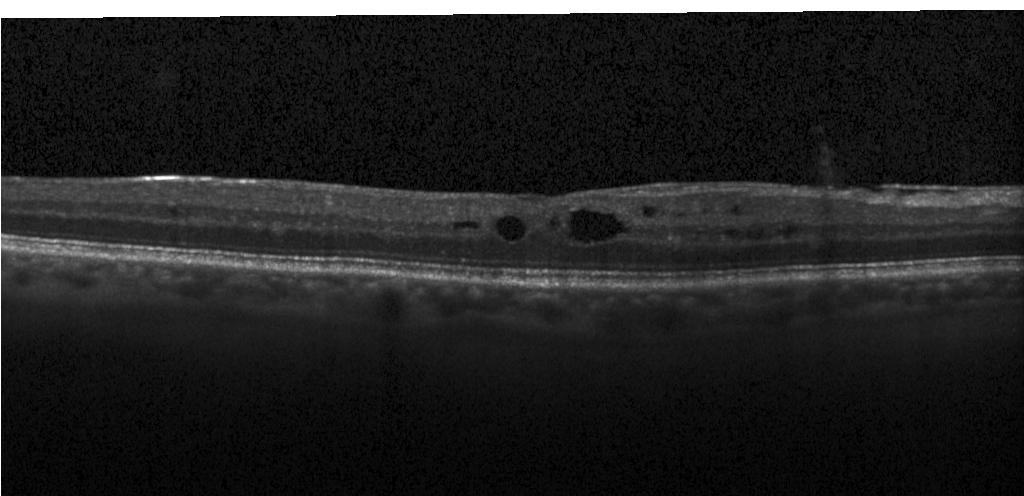 Optical coherence tomography B-scan — Finding: diabetic macular edema.